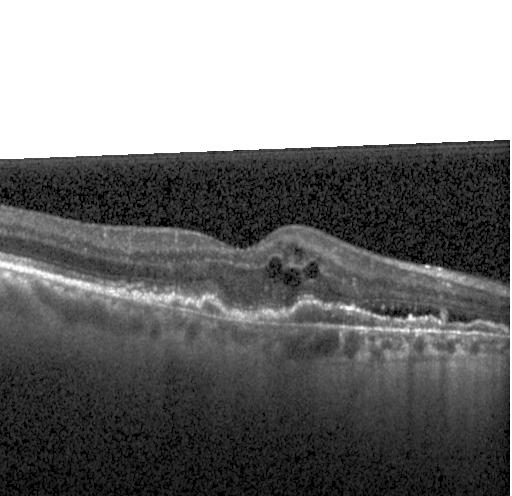 Macular OCT demonstrating choroidal neovascularization.